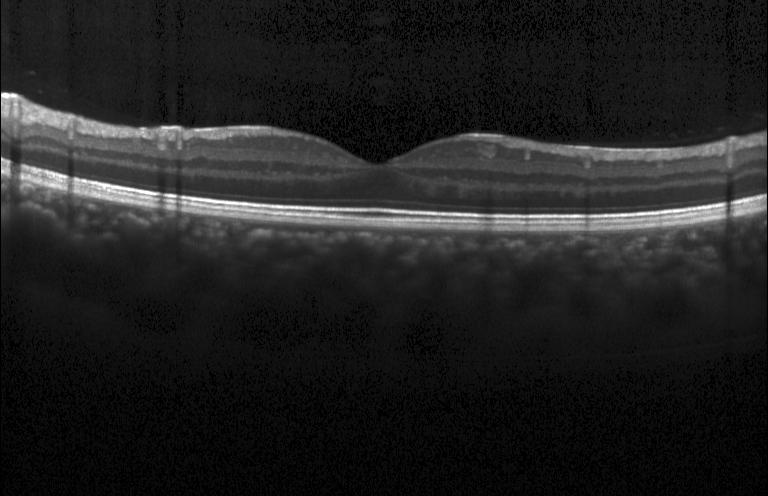

OCT line scan — Finding: no choroidal neovascularization, no diabetic macular edema, and no drusen.